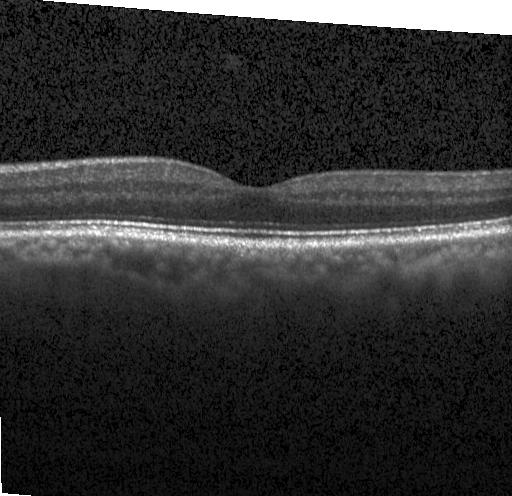

Optical coherence tomography scan.
OCT finding: no evidence of choroidal neovascularization, diabetic macular edema, or drusen.